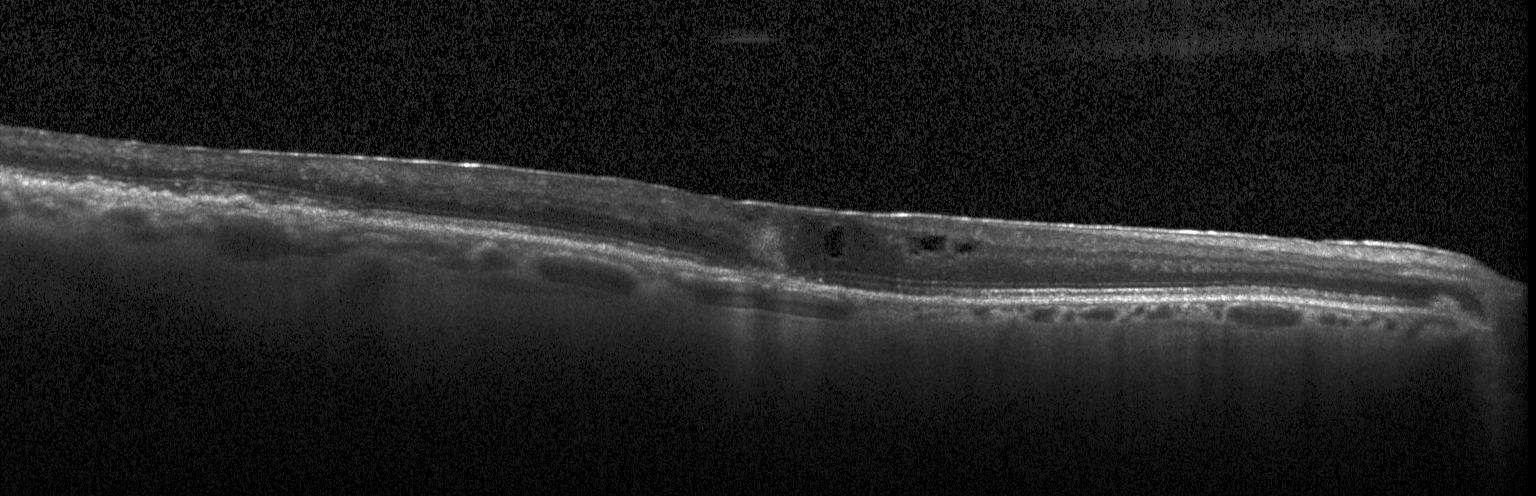
SD-OCT, horizontal scan through the fovea, OCT B-scan — This B-scan demonstrates a choroidal neovascular membrane.